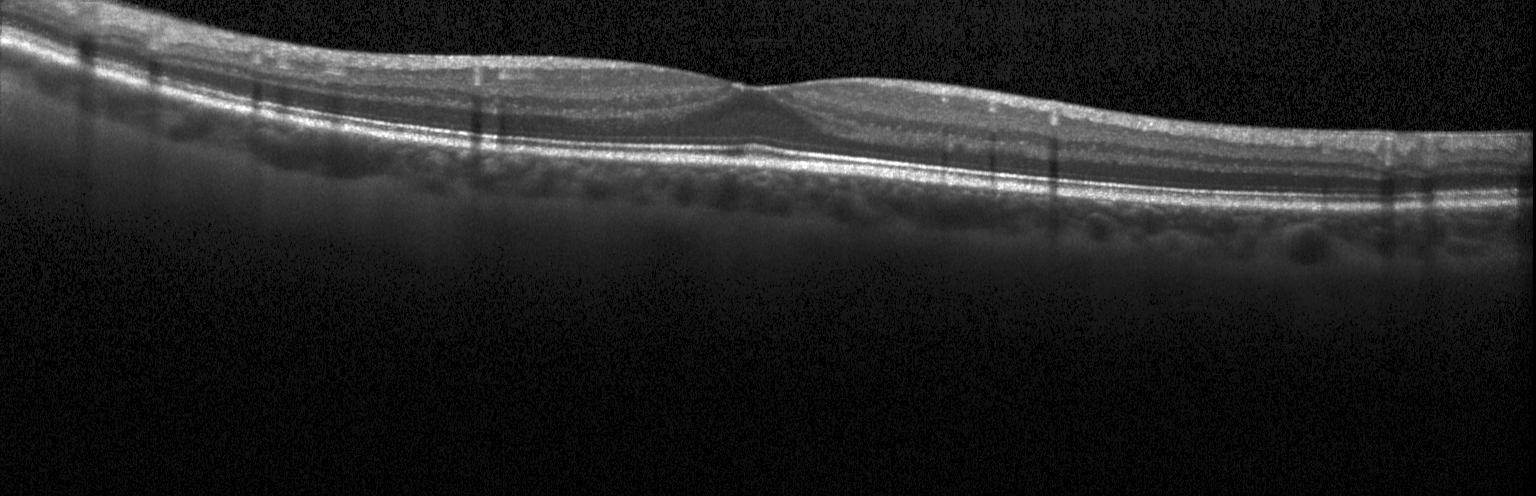

Instrument: Heidelberg Spectralis · through the macula · retinal OCT B-scan. Assessment: no CNV, no DME, and no drusen.